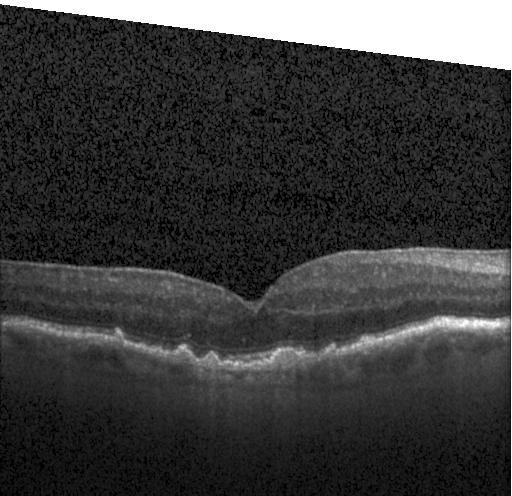 Dx: a choroidal neovascular membrane.